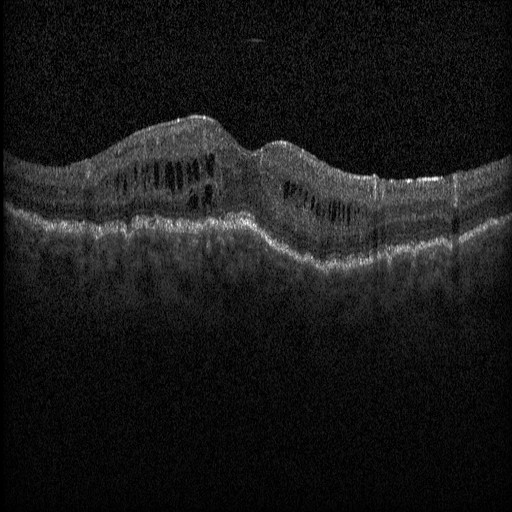

Spectral-domain OCT. Fovea-centered. OCT line scan
OCT finding: diabetic macular edema.